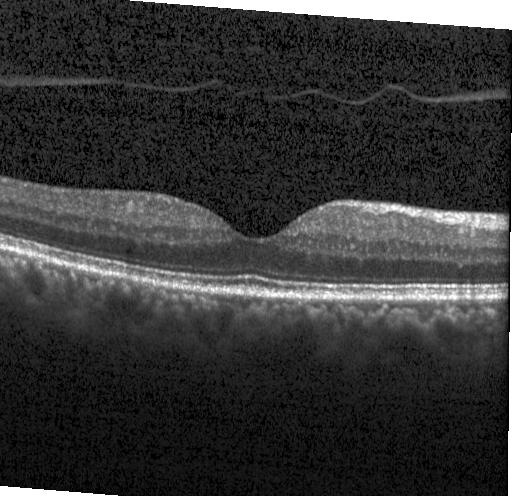 Macular scan · retinal OCT cross-section
Impression: no CNV, DME, or drusen.